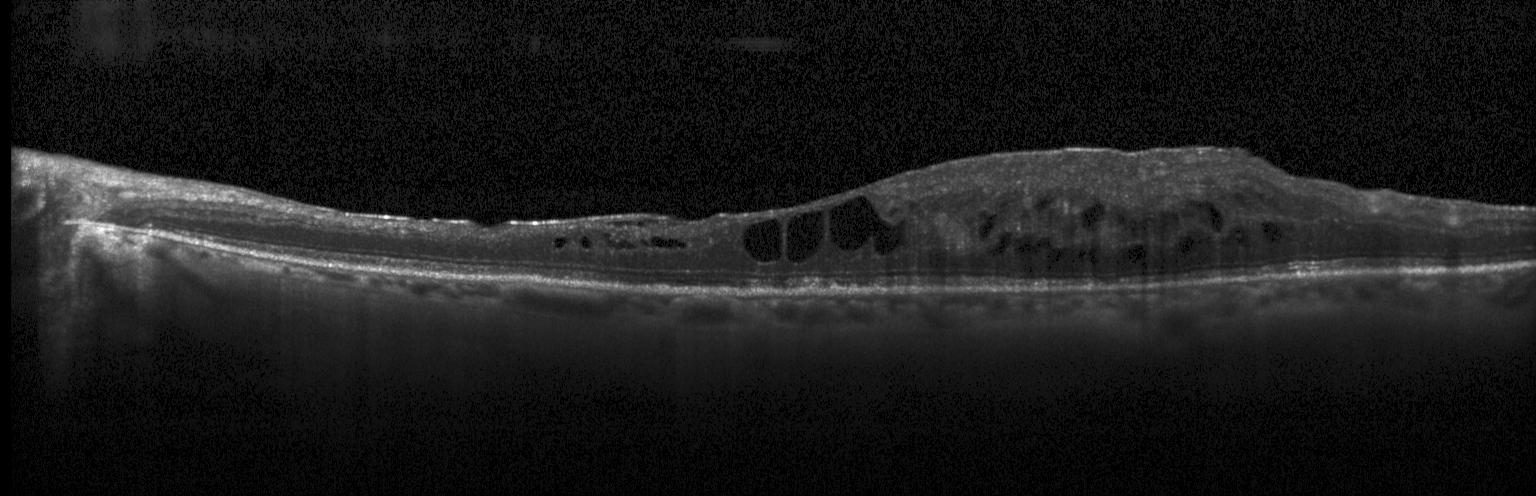 Acquired on a Heidelberg Spectralis; spectral-domain optical coherence tomography; retinal OCT B-scan; centered on the fovea.
OCT finding: diabetic macular edema (DME).